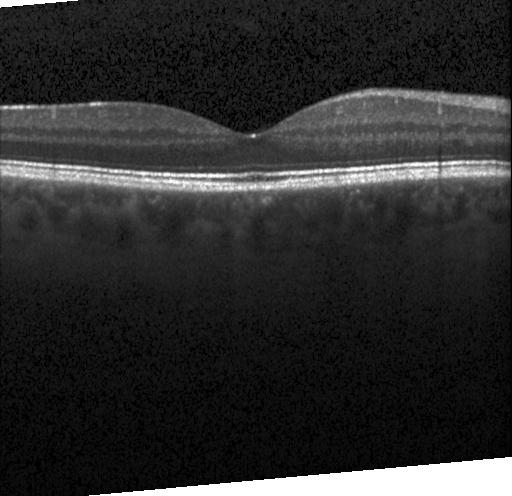

Horizontal scan through the fovea; SD-OCT; optical coherence tomography scan
Diagnosis: no evidence of choroidal neovascularization, diabetic macular edema, or drusen.